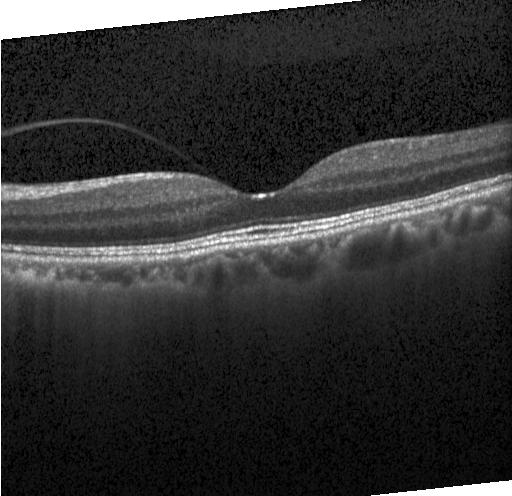 Acquired on a Heidelberg Spectralis. SD-OCT. Retinal OCT cross-section.
Impression: no choroidal neovascularization, no diabetic macular edema, and no drusen.